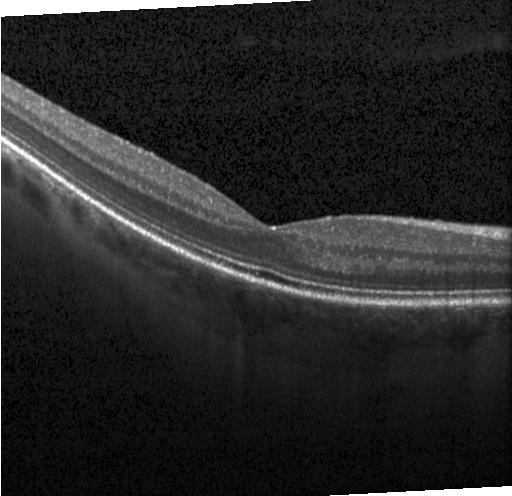

This B-scan demonstrates no choroidal neovascularization, diabetic macular edema, or drusen.